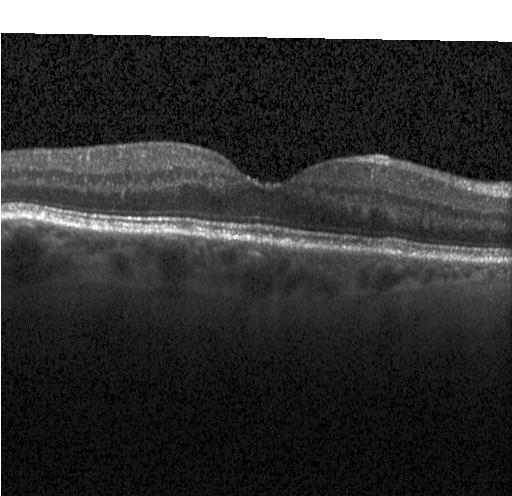

Optical coherence tomography B-scan, through the macula, SD-OCT. Assessment: neither CNV, DME, nor drusen.